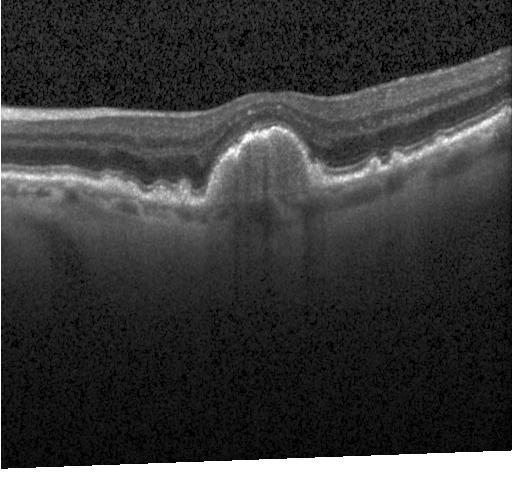 Spectral-domain optical coherence tomography · optical coherence tomography B-scan. Diagnosis: sub-RPE drusenoid deposits.